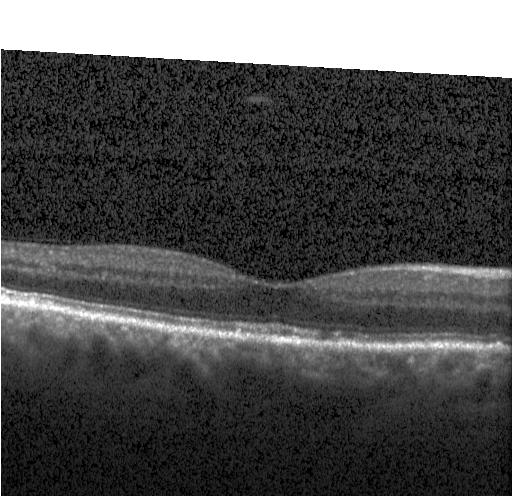

Optical coherence tomography scan. Centered on the fovea. Spectral-domain OCT
The scan shows no choroidal neovascularization, diabetic macular edema, or drusen.